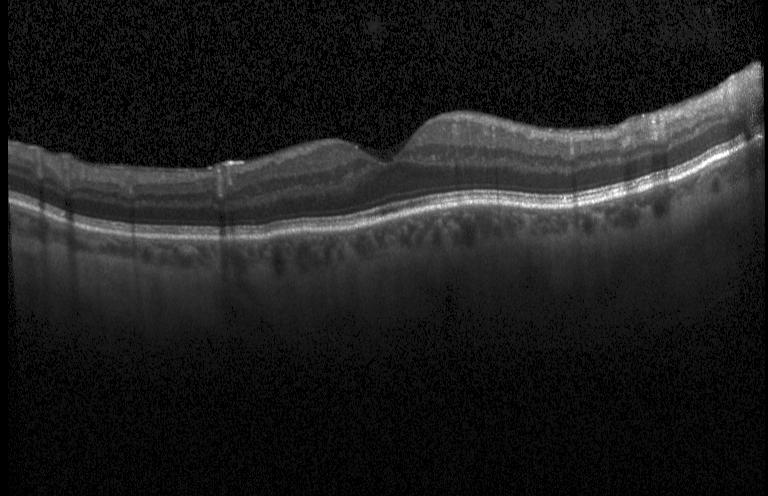 Assessment: no evidence of CNV, DME, or drusen.